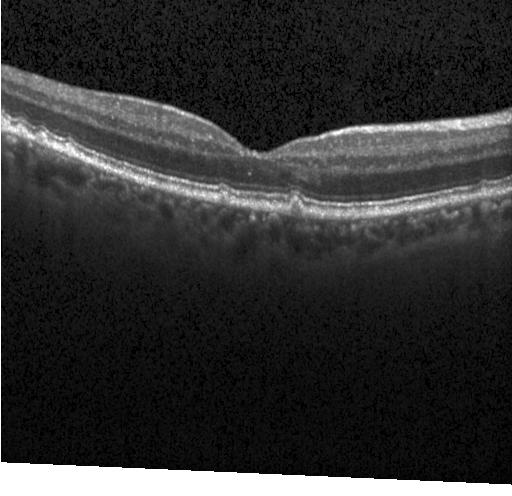 Spectral-domain optical coherence tomography, OCT line scan, fovea-centered
This B-scan demonstrates drusen.